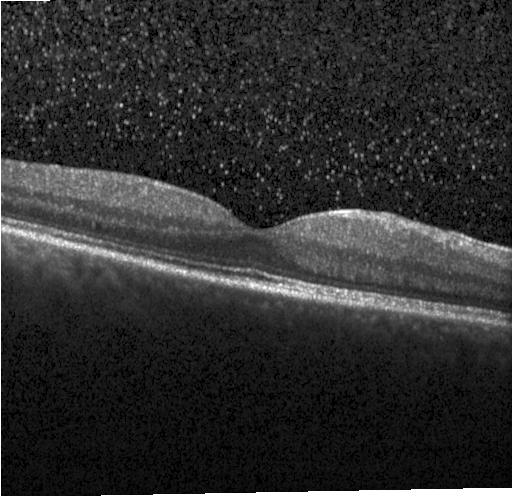

Assessment: no CNV, no DME, and no drusen.